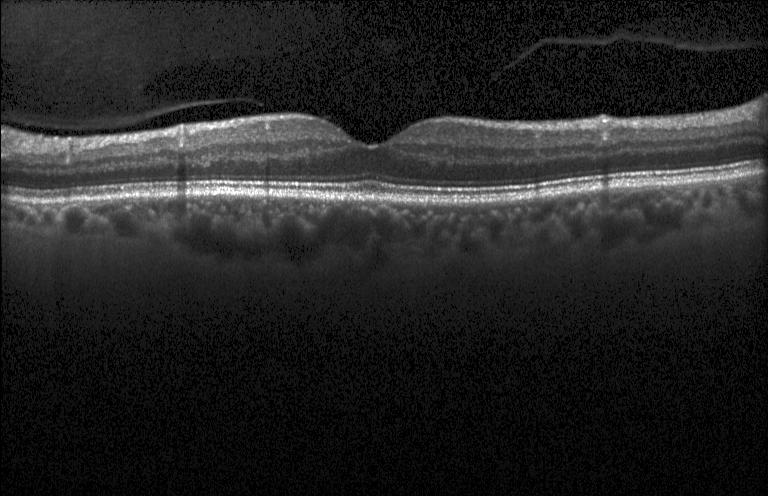

Optical coherence tomography B-scan — Assessment: no CNV, no DME, and no drusen.